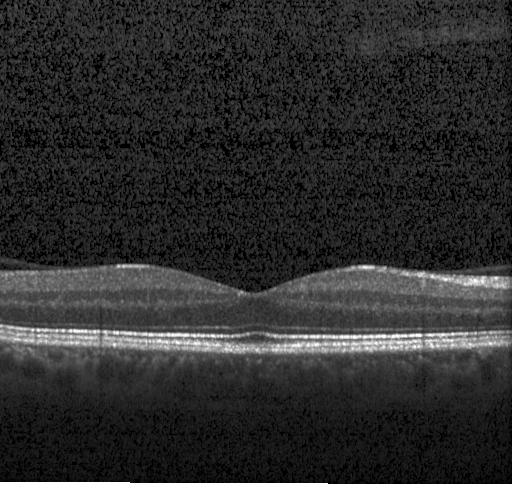

Acquired on a Heidelberg Spectralis · retinal OCT B-scan. Impression: no evidence of choroidal neovascularization, diabetic macular edema, or drusen.